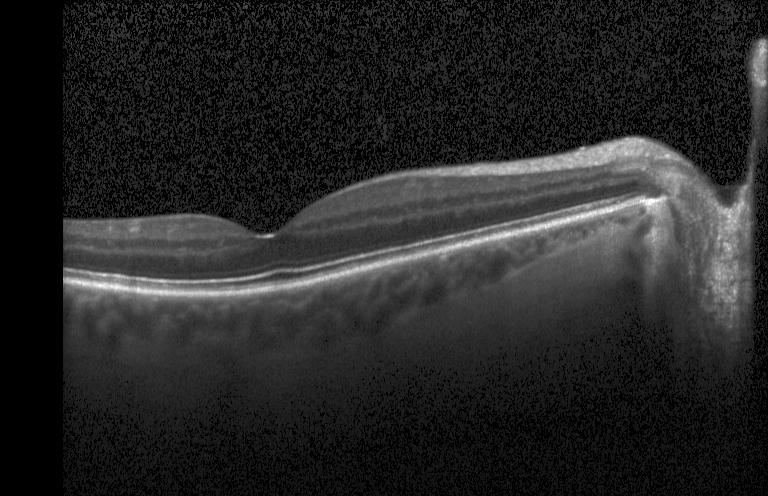
Heidelberg Spectralis OCT system. Optical coherence tomography scan. Macular OCT: neither choroidal neovascularization, diabetic macular edema, nor drusen.